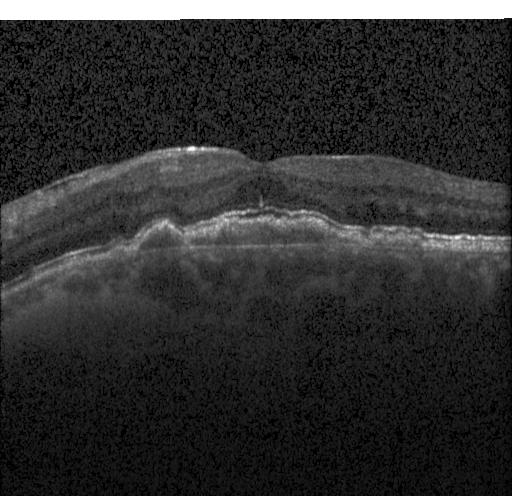
OCT line scan. Spectral-domain OCT. Acquired on a Heidelberg Spectralis. This B-scan demonstrates a choroidal neovascular membrane.